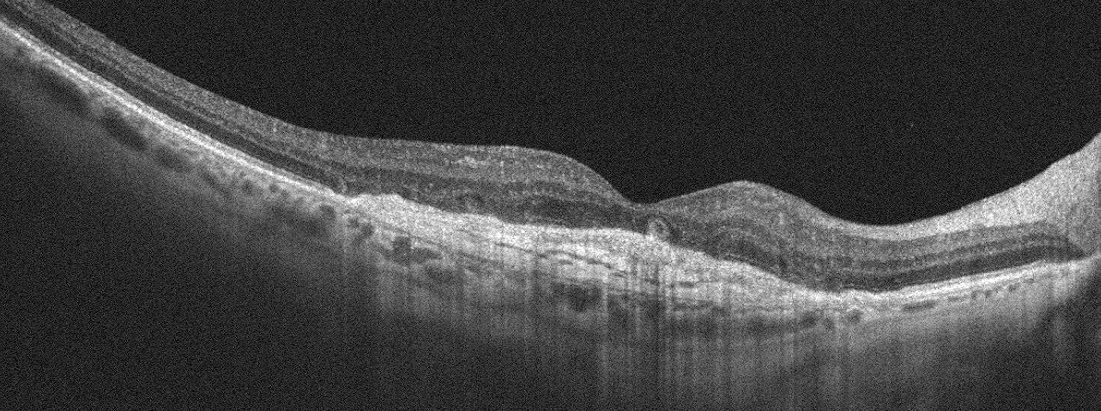 Spectral-domain OCT B-scan: AMD.